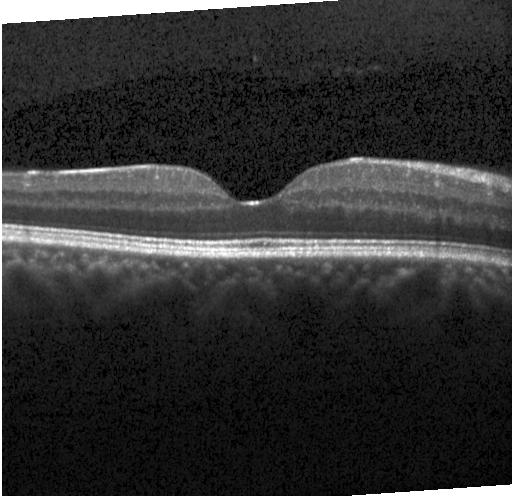

Acquired on a Heidelberg Spectralis · OCT line scan · SD-OCT · macular scan.
Assessment: no evidence of choroidal neovascularization, diabetic macular edema, or drusen.